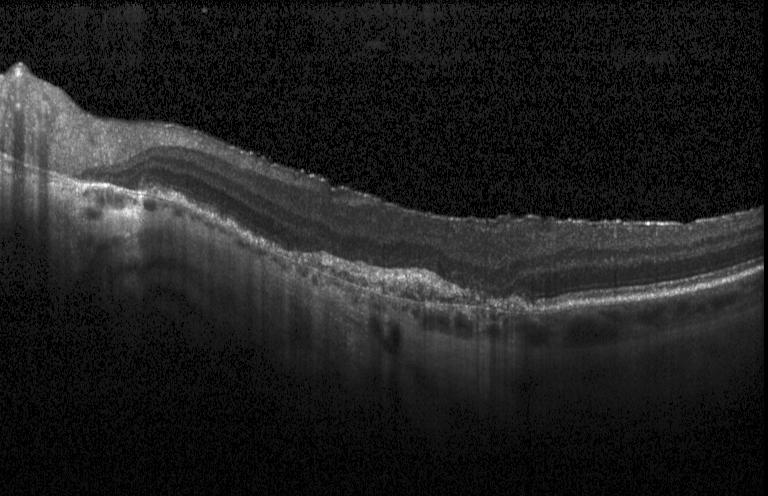 OCT line scan.
This B-scan demonstrates a choroidal neovascular membrane.